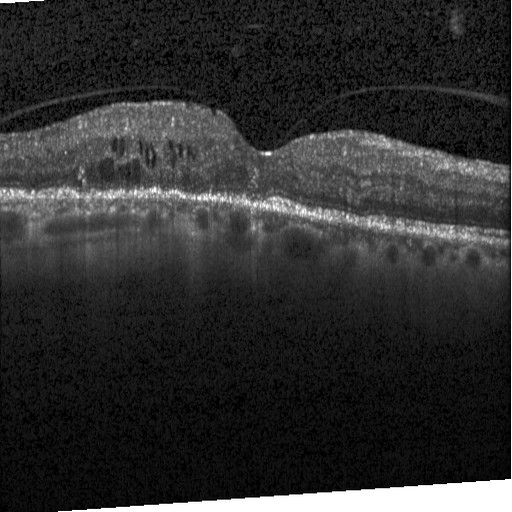

Spectral-domain OCT; centered on the fovea; retinal OCT cross-section; Heidelberg Spectralis — Assessment: DME.